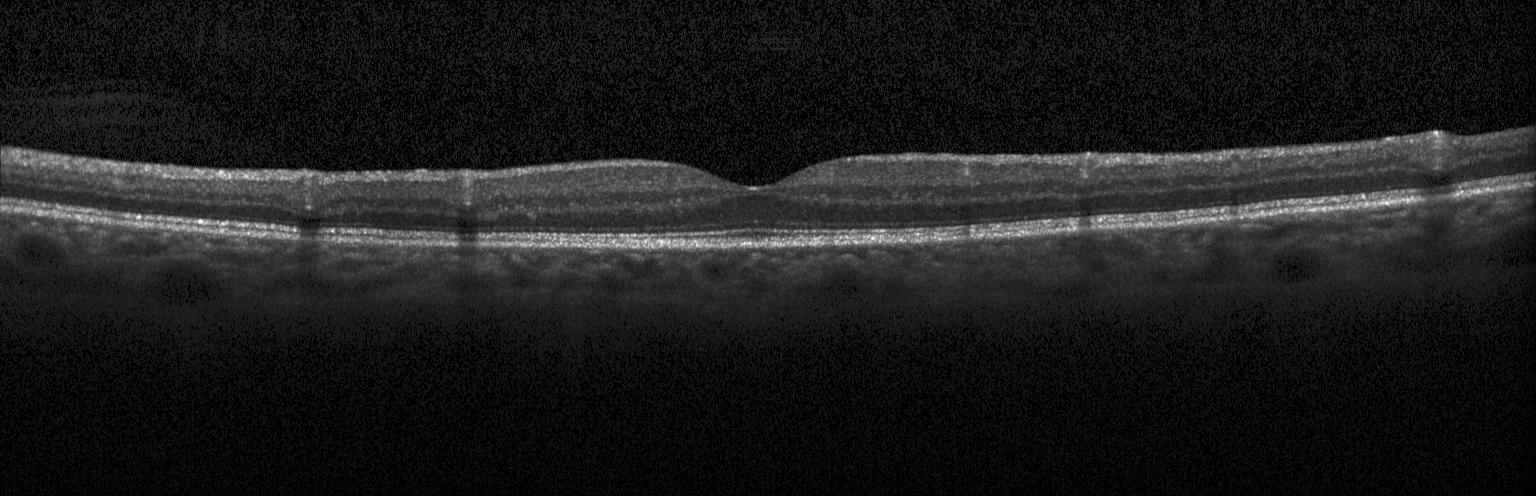 Optical coherence tomography B-scan. SD-OCT. Macular scan — Impression: no choroidal neovascularization, no diabetic macular edema, and no drusen.